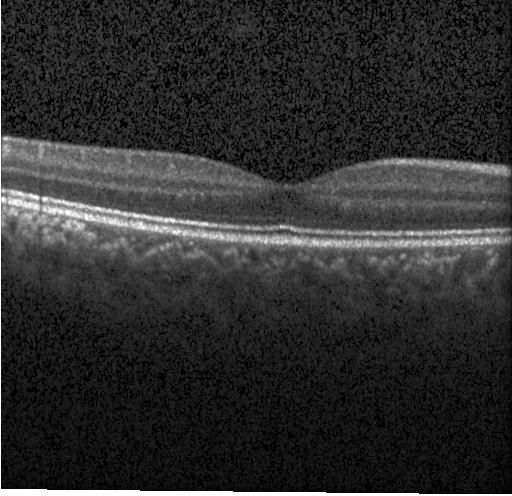

Heidelberg Spectralis; centered on the fovea; spectral-domain optical coherence tomography; OCT B-scan
Impression: neither choroidal neovascularization, diabetic macular edema, nor drusen.